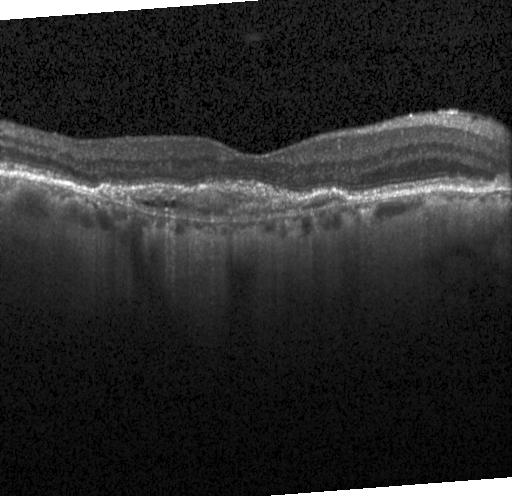
OCT scan showing choroidal neovascularization.